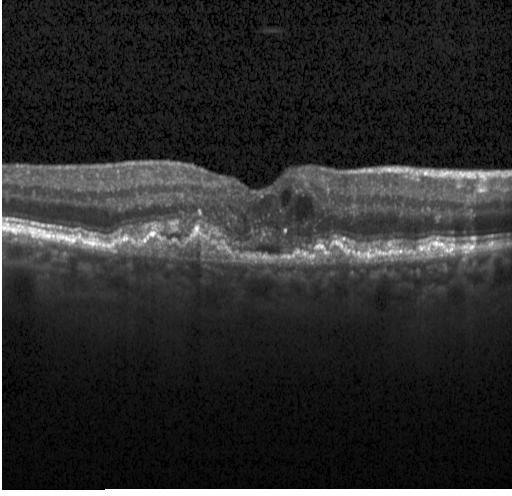
Retinal OCT cross-section, spectral-domain OCT, horizontal scan through the fovea. Impression: a choroidal neovascular membrane.